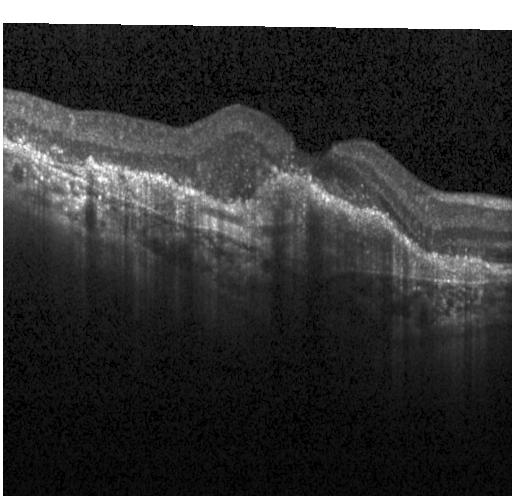

Diagnosis: choroidal neovascularization (CNV).